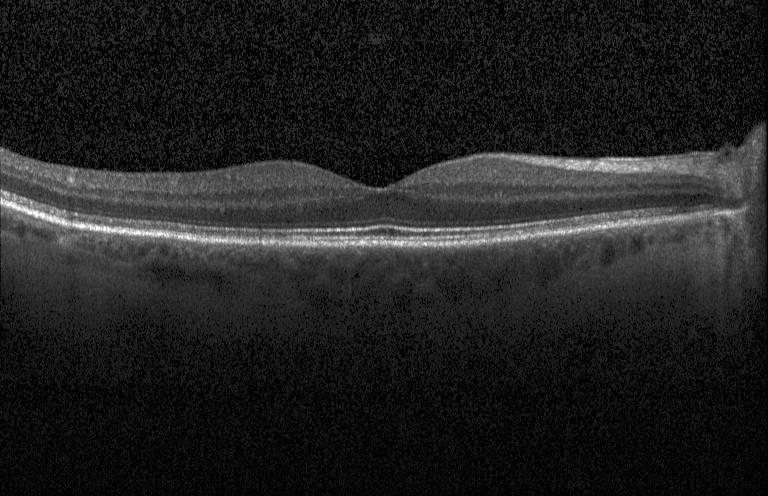 Retinal OCT cross-section showing no choroidal neovascularization, diabetic macular edema, or drusen.